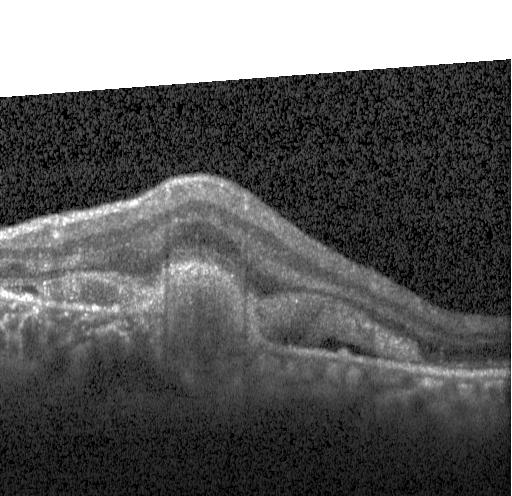 Acquired on a Heidelberg Spectralis, spectral-domain OCT, horizontal scan through the fovea, OCT line scan
Diagnosis: choroidal neovascularization.